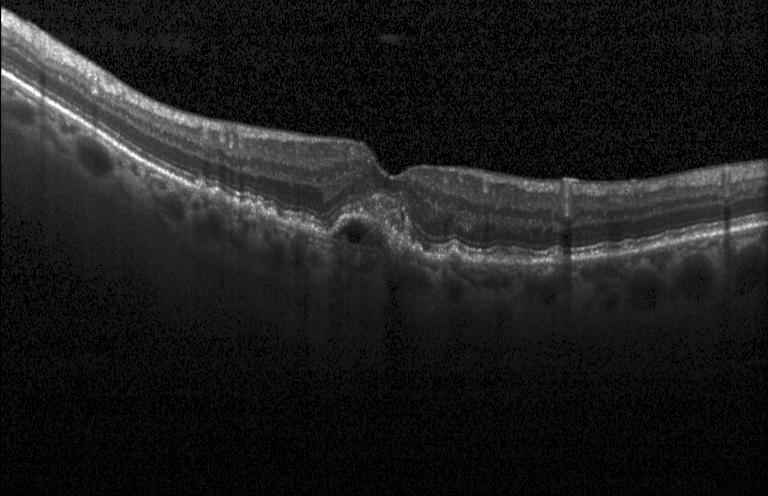 Optical coherence tomography B-scan.
Finding: choroidal neovascularization.